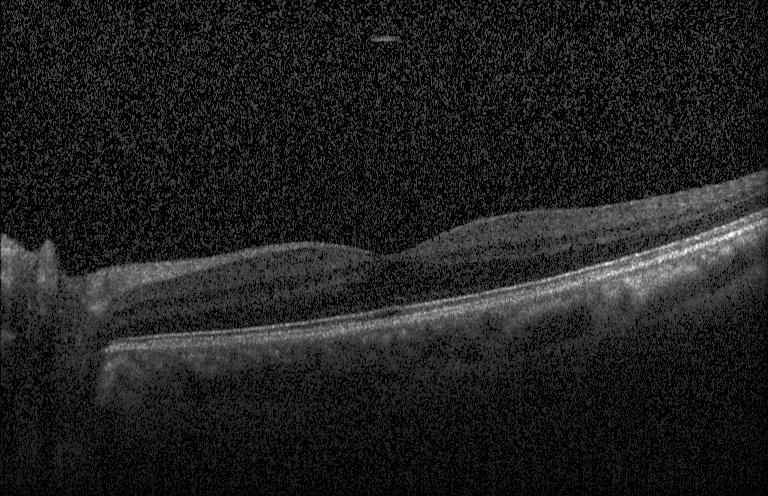
OCT finding: no CNV, no DME, and no drusen.